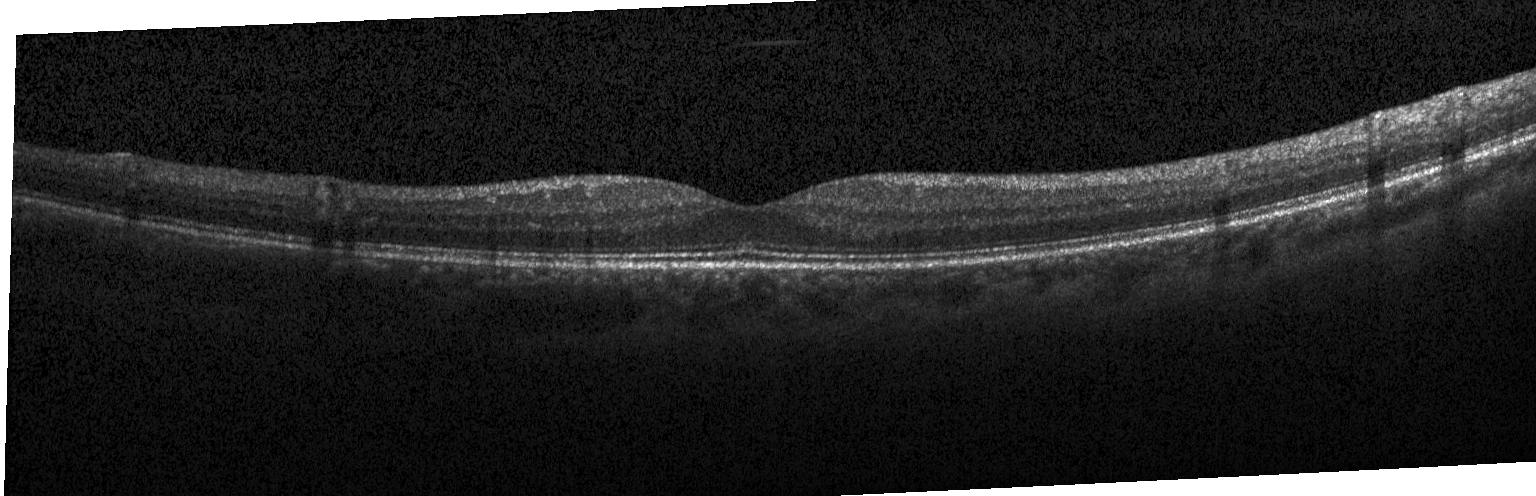 Retinal OCT cross-section, spectral-domain optical coherence tomography, acquired on a Heidelberg Spectralis
Dx: no CNV, no DME, and no drusen.